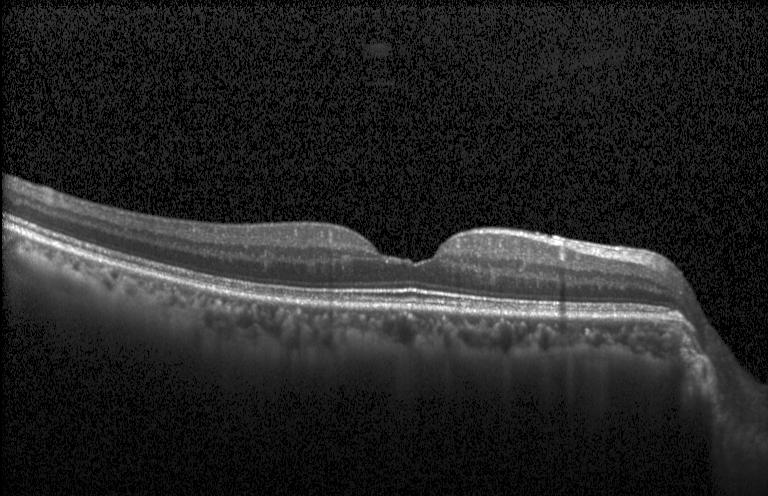
Instrument: Heidelberg Spectralis. Retinal OCT cross-section
Finding: neither choroidal neovascularization, diabetic macular edema, nor drusen.